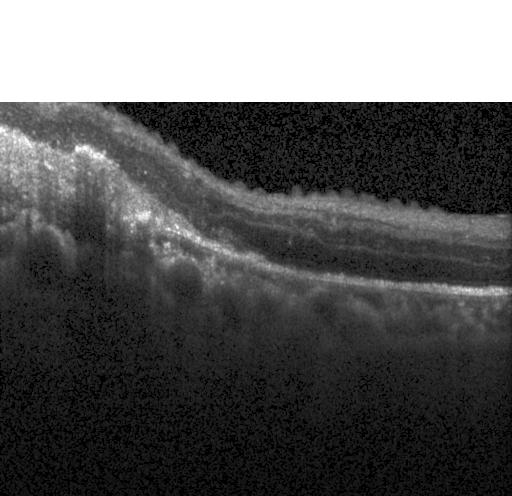
Through the macula, OCT line scan, spectral-domain OCT, Heidelberg Spectralis.
The scan shows a choroidal neovascular membrane.